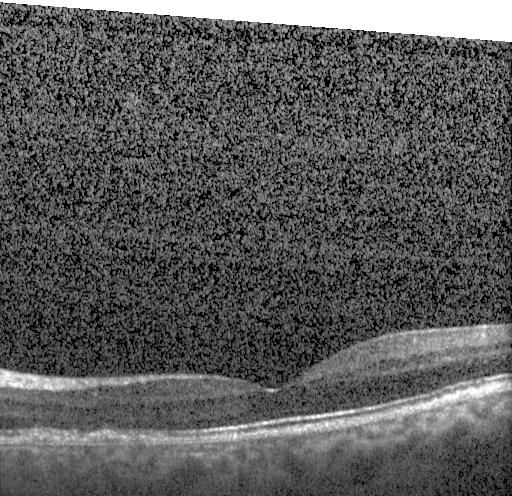

Retinal OCT cross-section. Fovea-centered. Finding: a choroidal neovascular membrane.